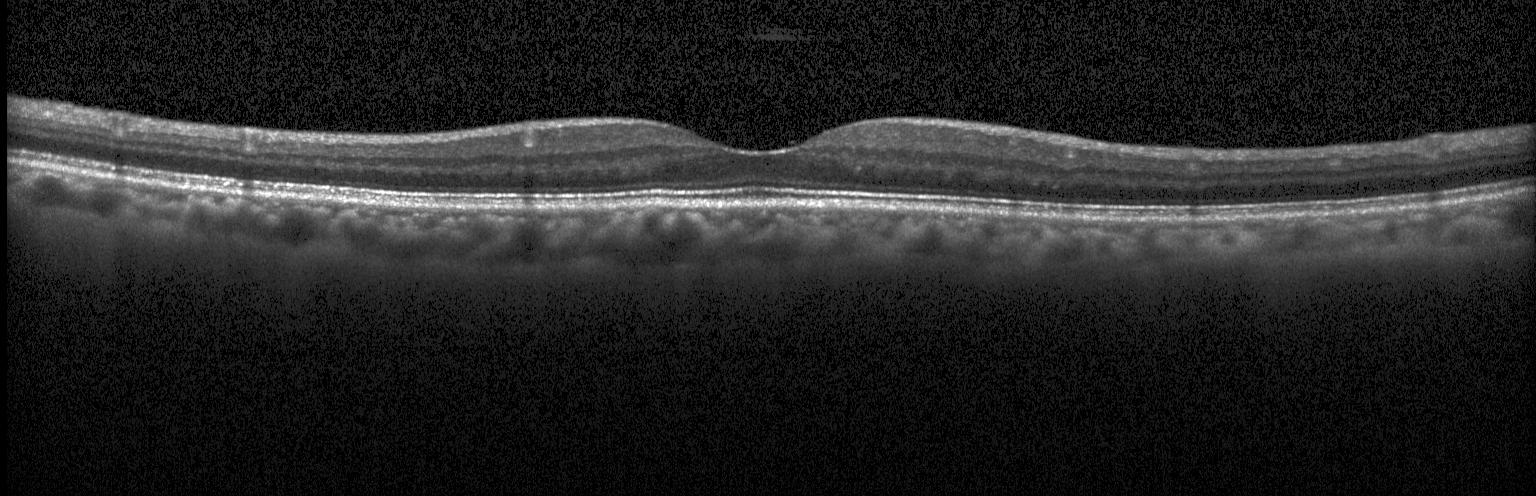 No choroidal neovascularization, no diabetic macular edema, and no drusen.